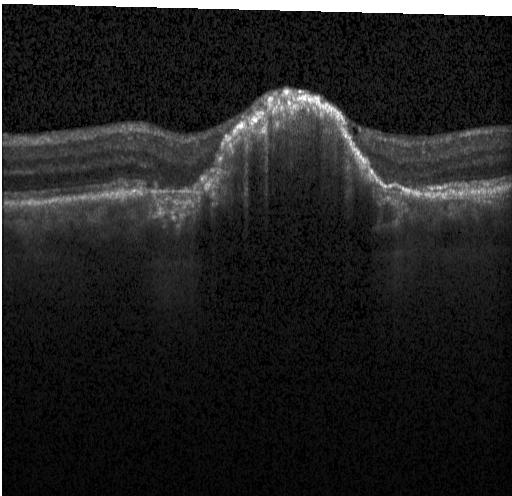
Optical coherence tomography scan, centered on the fovea, instrument: Heidelberg Spectralis.
Assessment: choroidal neovascularization.